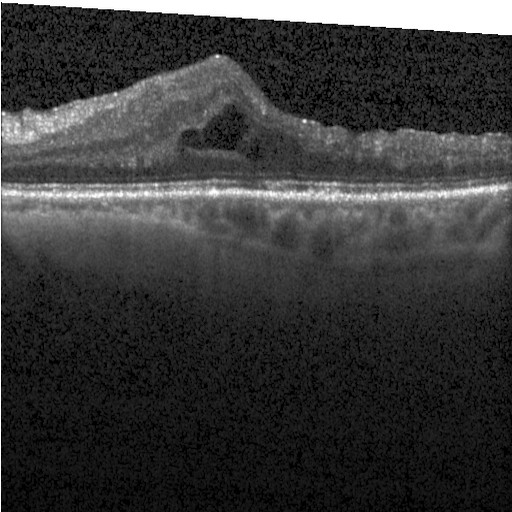

Retinal OCT B-scan. Finding: diabetic macular edema.